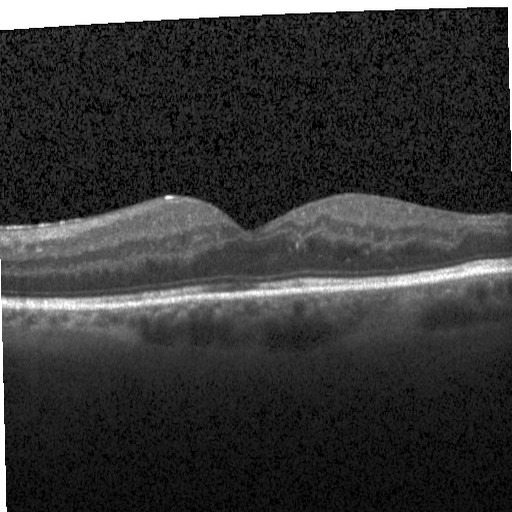
Diagnosis: diabetic macular edema.